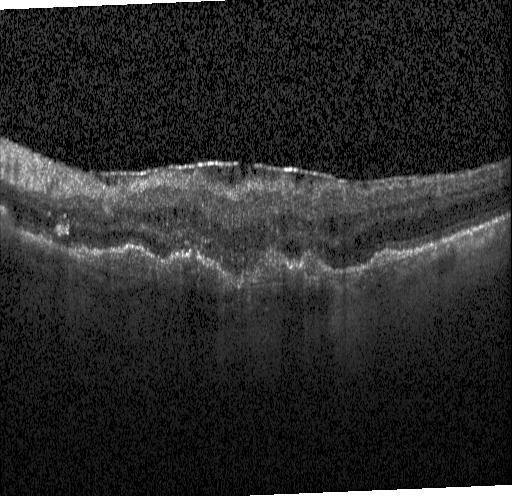
Spectral-domain OCT. Optical coherence tomography scan. Horizontal scan through the fovea. Macular OCT: choroidal neovascularization (CNV).